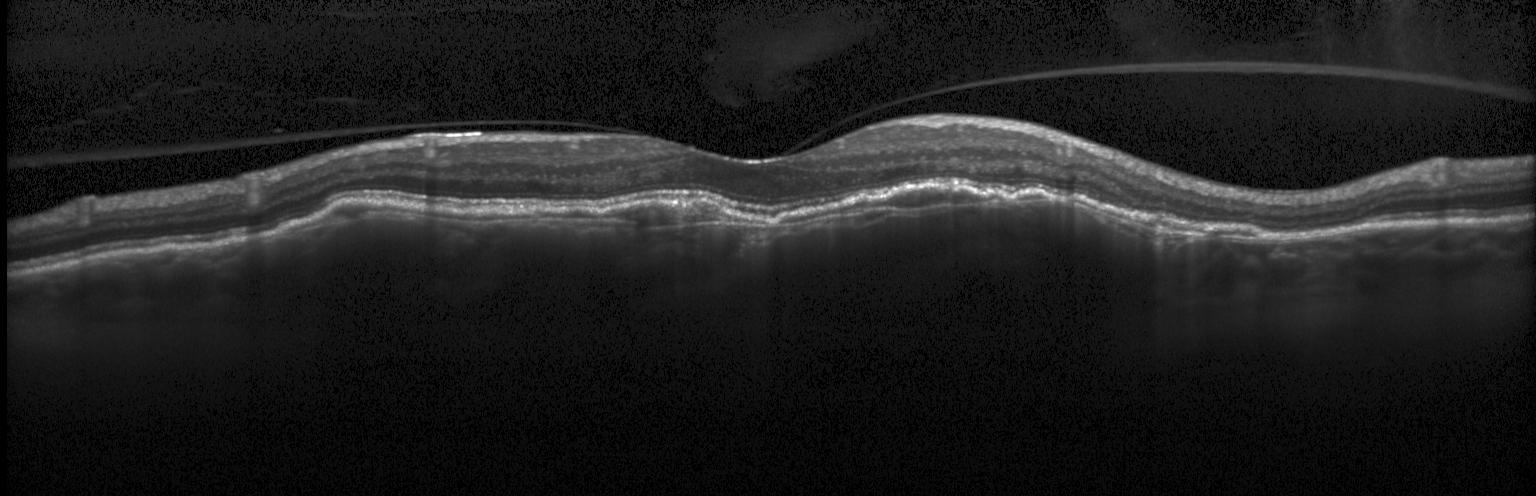
OCT B-scan; through the macula
Assessment: choroidal neovascularization.